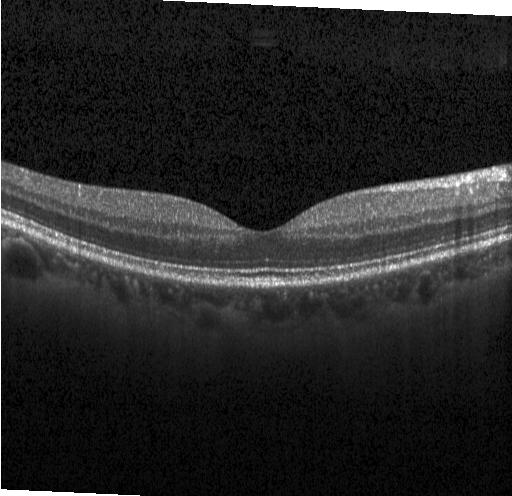
Spectral-domain OCT · through the macula · Heidelberg Spectralis OCT system · OCT line scan. Dx: no evidence of choroidal neovascularization, diabetic macular edema, or drusen.